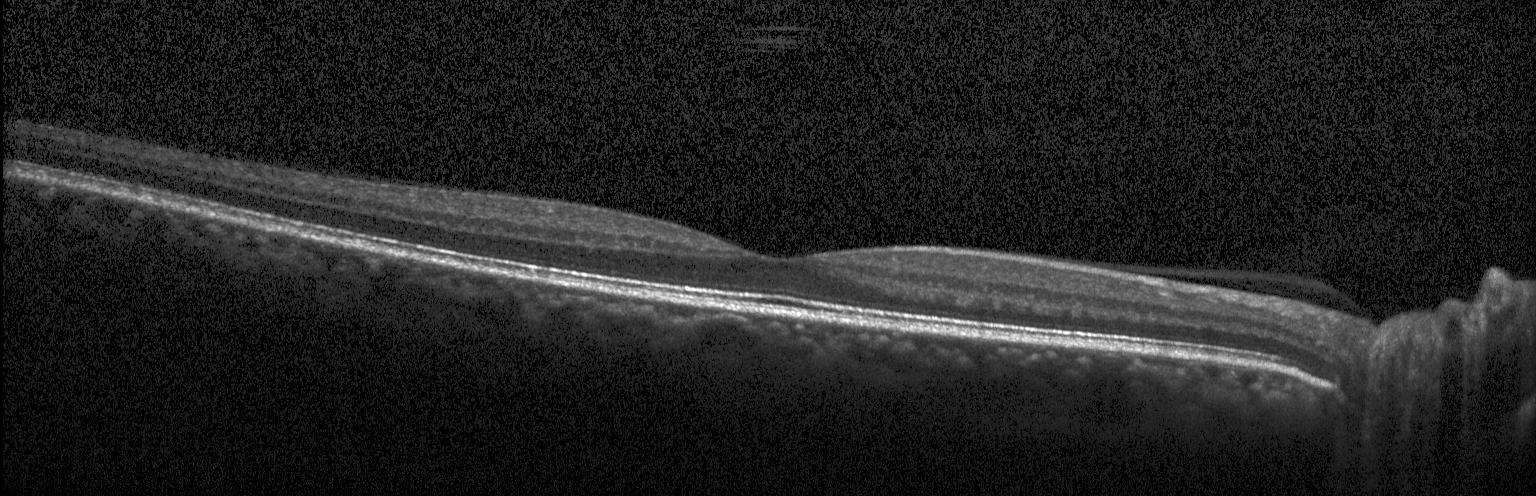

Neither choroidal neovascularization, diabetic macular edema, nor drusen.